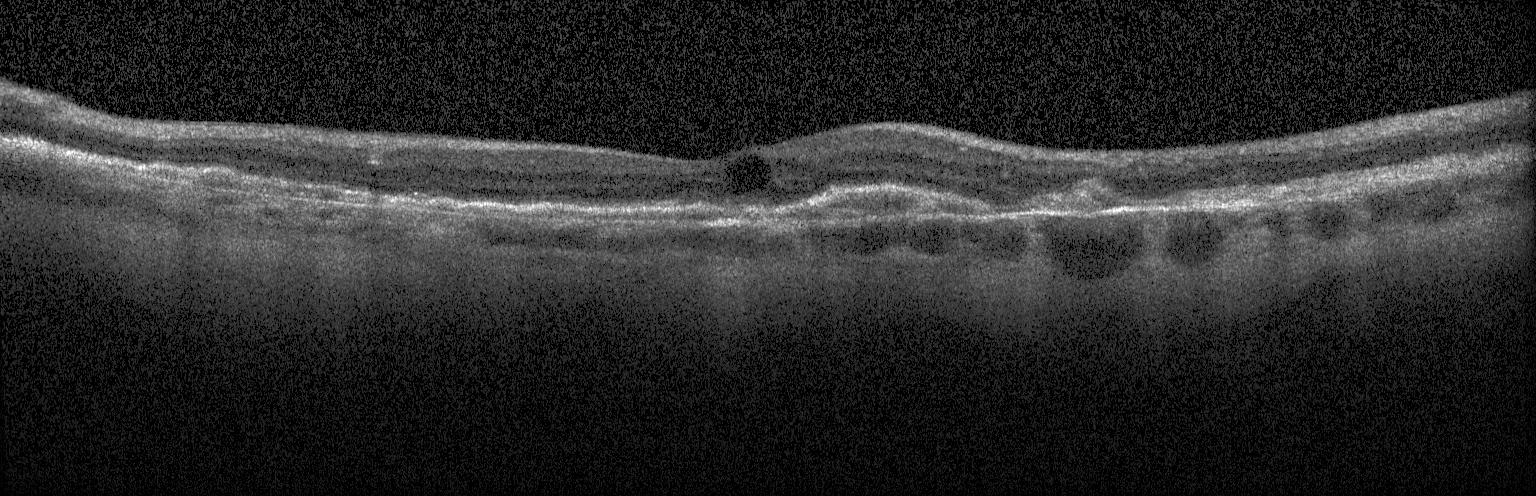 Impression: a choroidal neovascular membrane.